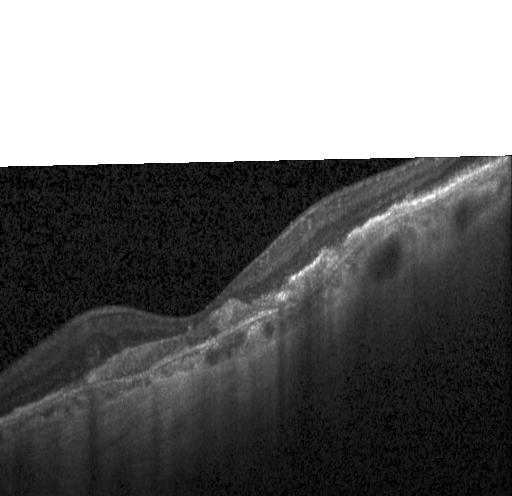
OCT scan showing choroidal neovascularization (CNV).